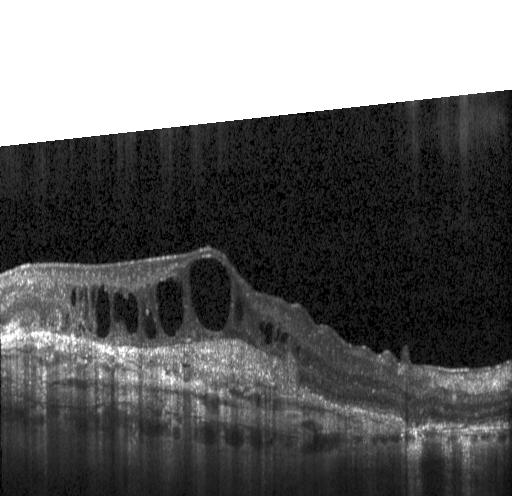

Diagnosis: a choroidal neovascular membrane.